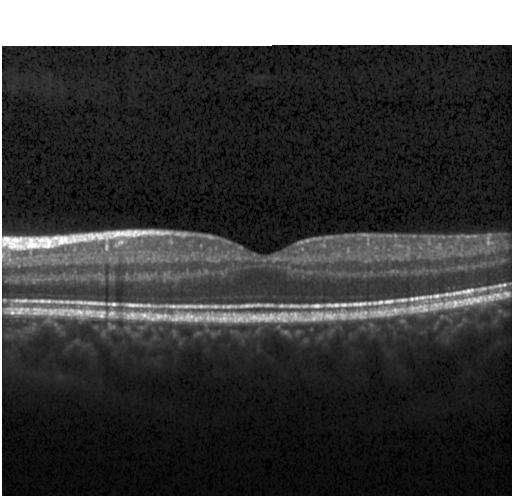 Retinal OCT cross-section; centered on the fovea — Dx: neither CNV, DME, nor drusen.